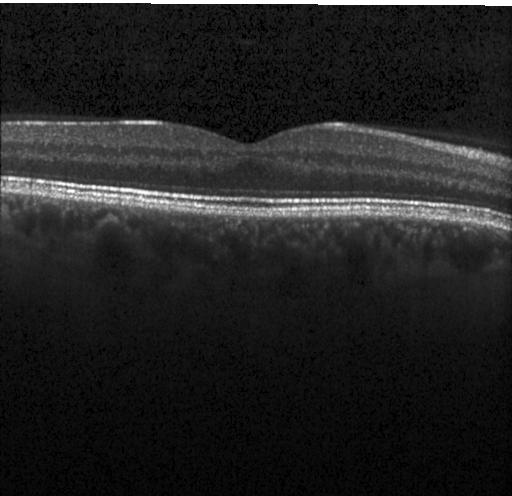 Assessment: no CNV, DME, or drusen.